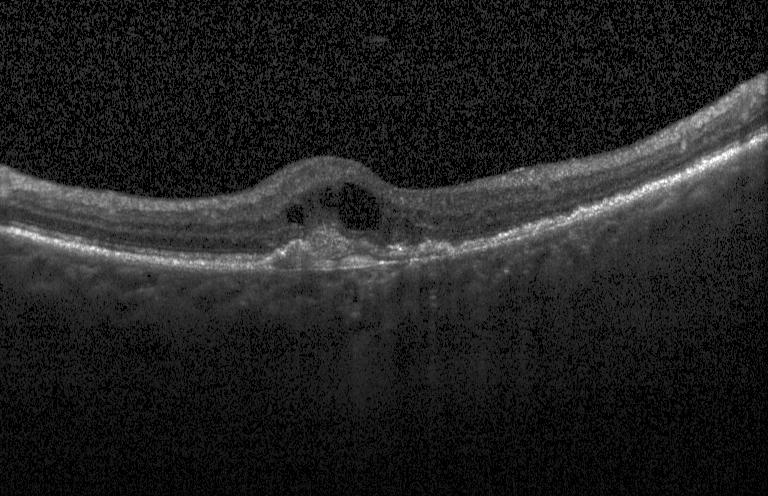 OCT B-scan showing a choroidal neovascular membrane.